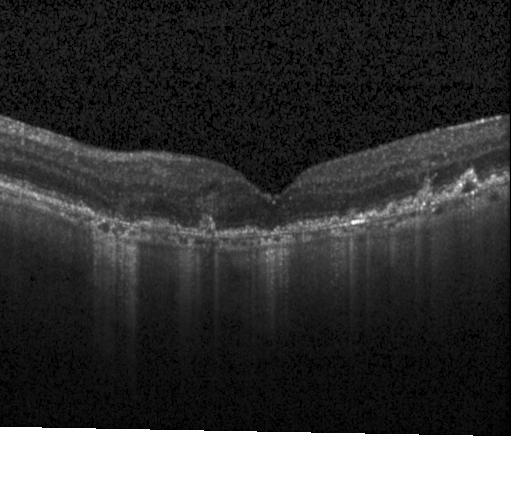 Heidelberg Spectralis OCT system; optical coherence tomography B-scan.
Macular OCT: CNV.